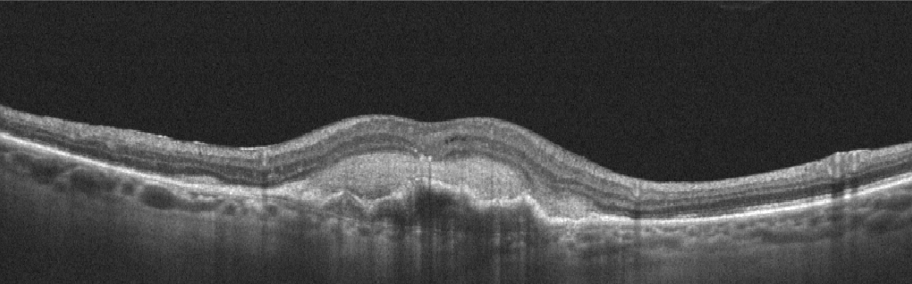
OCT line scan; Optovue Avanti RTVue XR; through the macula
Assessment: AMD.